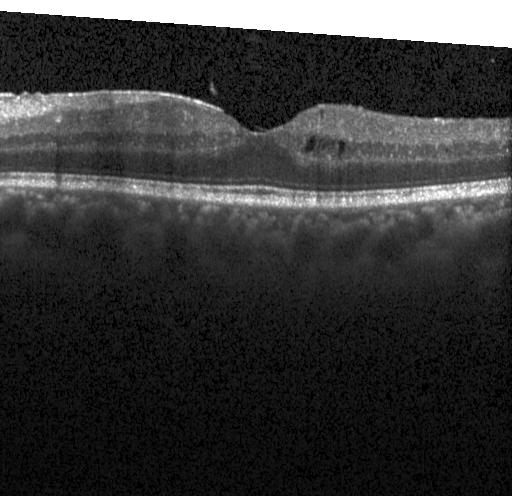 Impression: diabetic macular edema (DME).